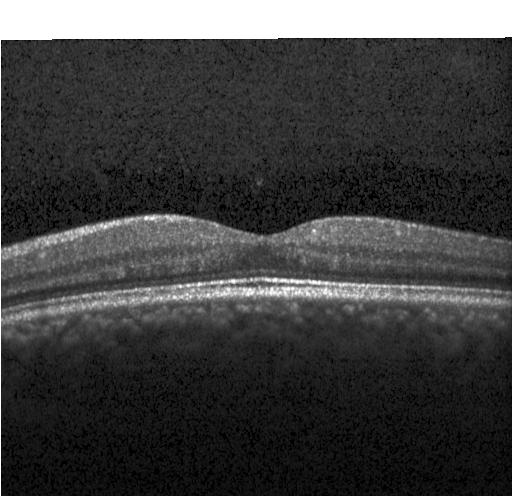

Optical coherence tomography scan
Neither CNV, DME, nor drusen.